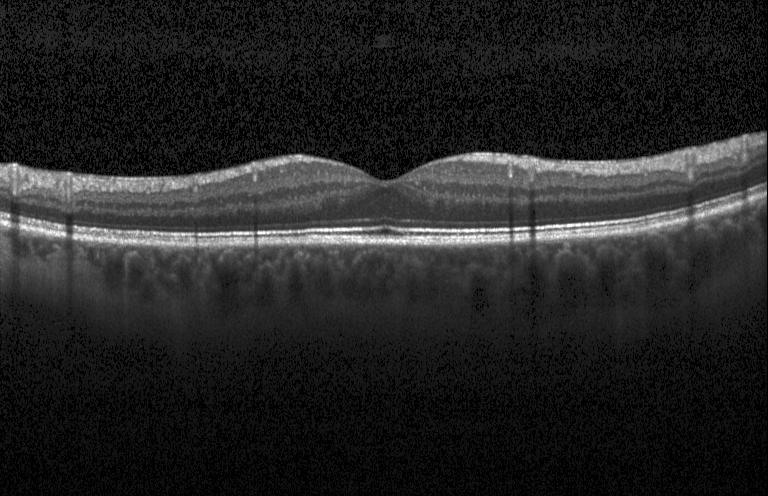 Optical coherence tomography scan. Through the macula. Macular OCT: no CNV, no DME, and no drusen.